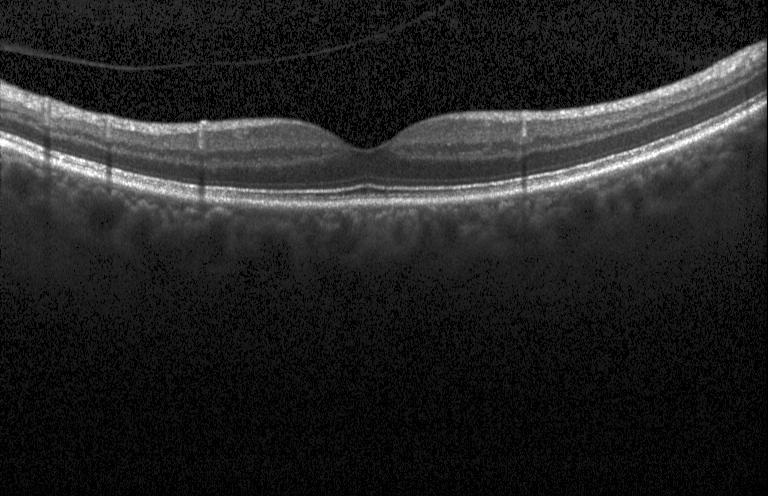
Finding: no CNV, no DME, and no drusen.